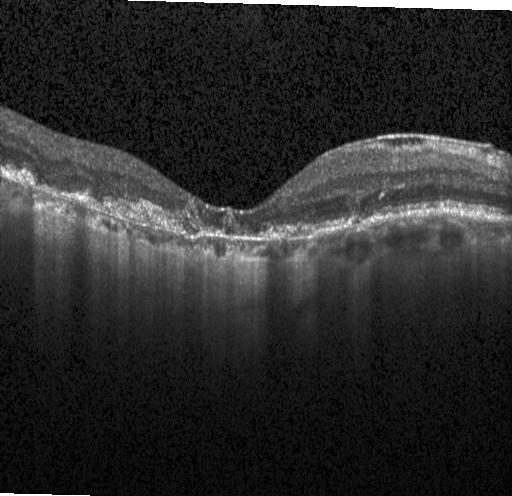
Diagnosis: choroidal neovascularization (CNV).